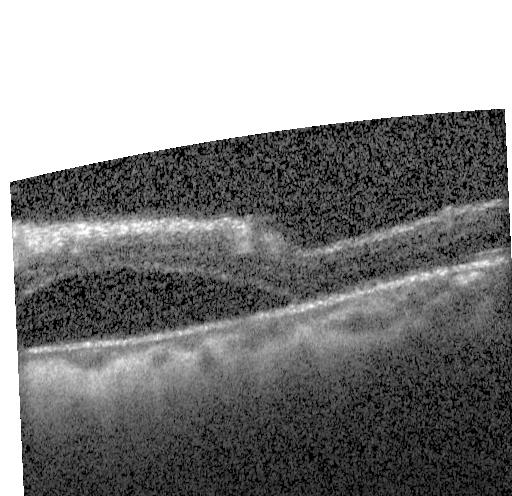

Heidelberg Spectralis OCT system. OCT B-scan
Impression: CNV.